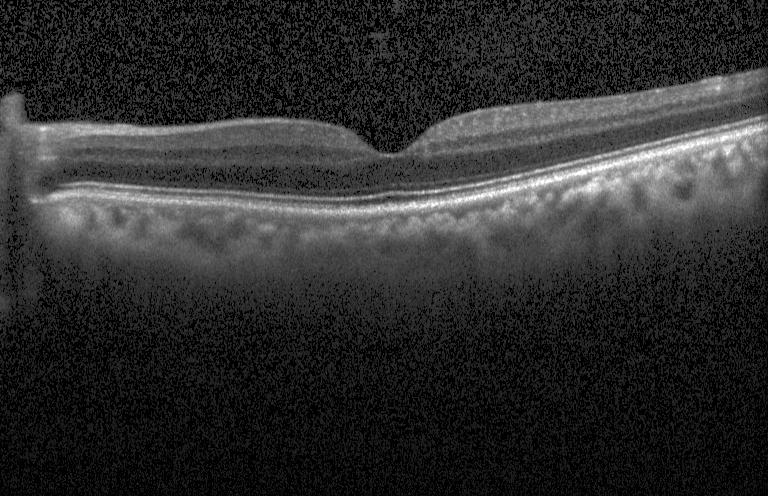 Macular OCT: no choroidal neovascularization, diabetic macular edema, or drusen.